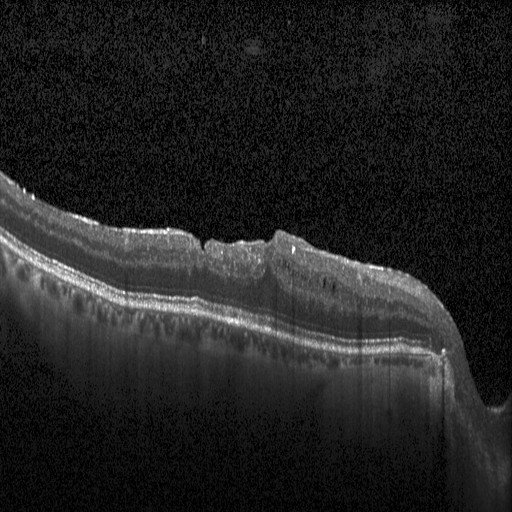
The scan shows DME.